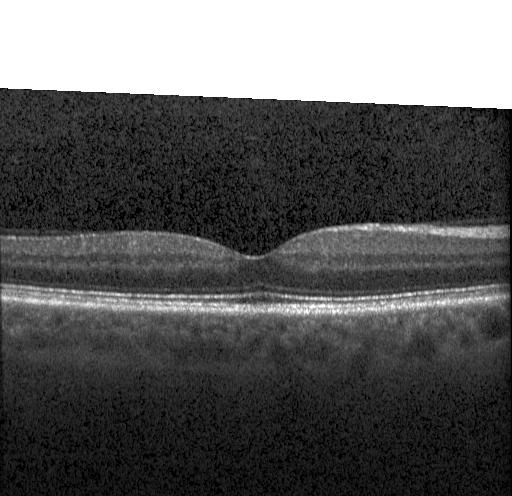
Retinal OCT cross-section. Spectral-domain OCT. Through the macula — Impression: no choroidal neovascularization, diabetic macular edema, or drusen.